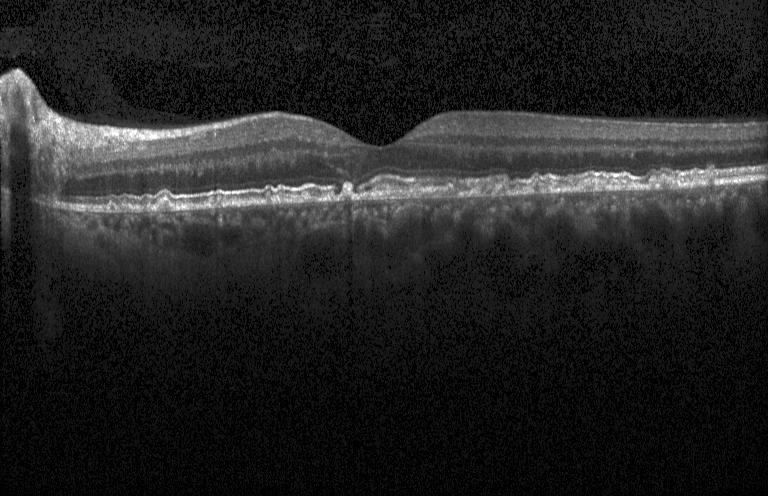
OCT B-scan showing multiple drusen.